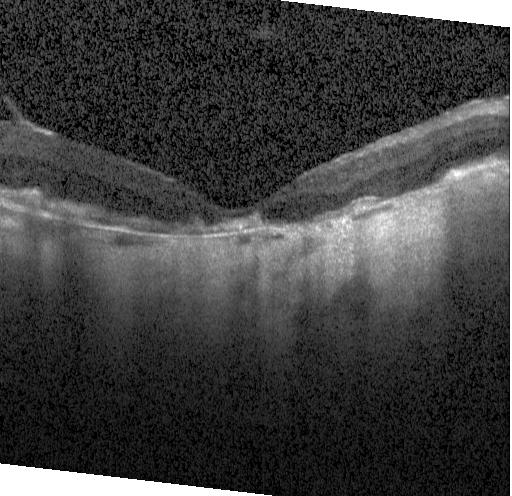
Retinal OCT cross-section, Heidelberg Spectralis, macular scan — Finding: choroidal neovascularization (CNV).